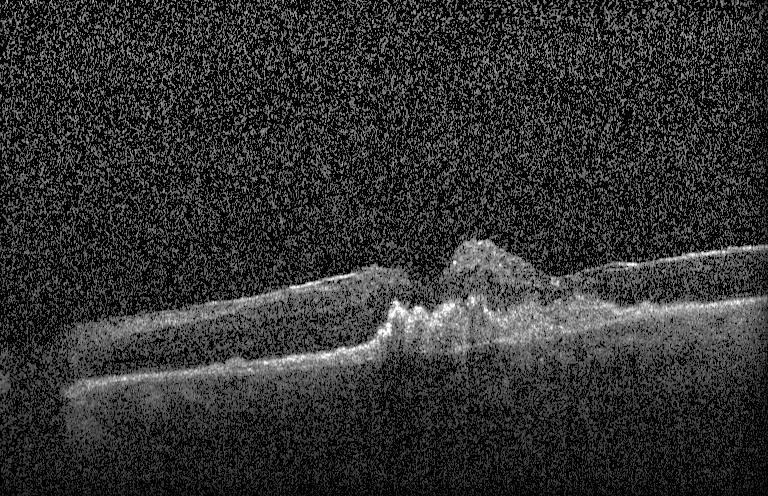
Retinal OCT cross-section; macular scan — Impression: choroidal neovascularization.